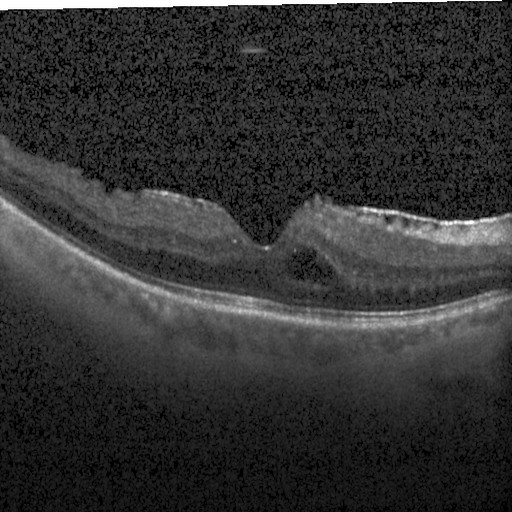

Instrument: Heidelberg Spectralis · optical coherence tomography B-scan · macular scan · spectral-domain OCT
Diagnosis: DME.